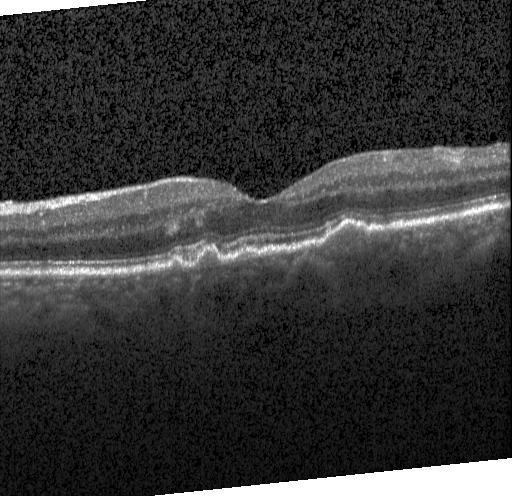

Heidelberg Spectralis OCT system · spectral-domain OCT · optical coherence tomography B-scan. The scan shows sub-RPE drusenoid deposits.